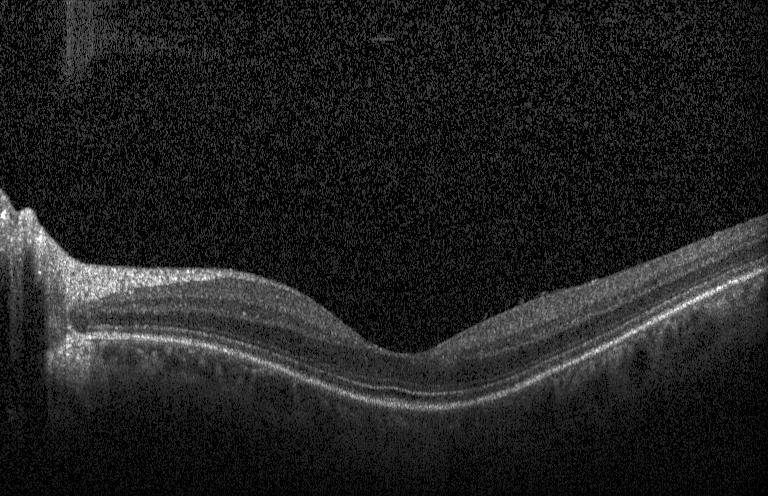

This B-scan demonstrates no choroidal neovascularization, diabetic macular edema, or drusen.